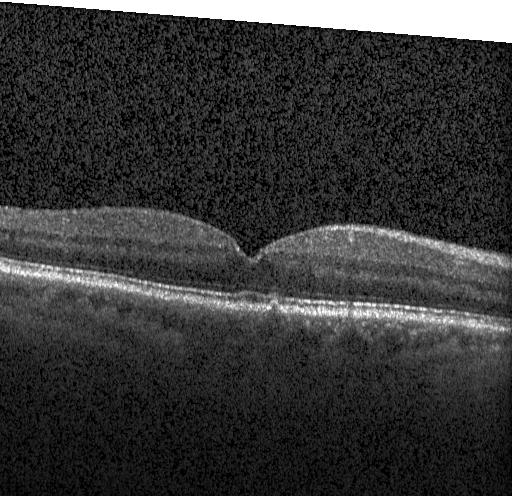 Retinal OCT B-scan. Macular OCT: sub-RPE drusenoid deposits.